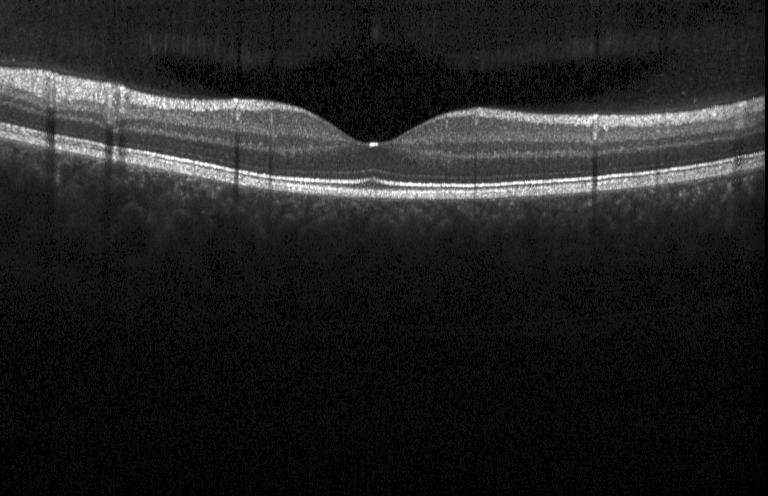

Instrument: Heidelberg Spectralis. Fovea-centered. Retinal OCT cross-section. Spectral-domain optical coherence tomography.
The scan shows no evidence of choroidal neovascularization, diabetic macular edema, or drusen.